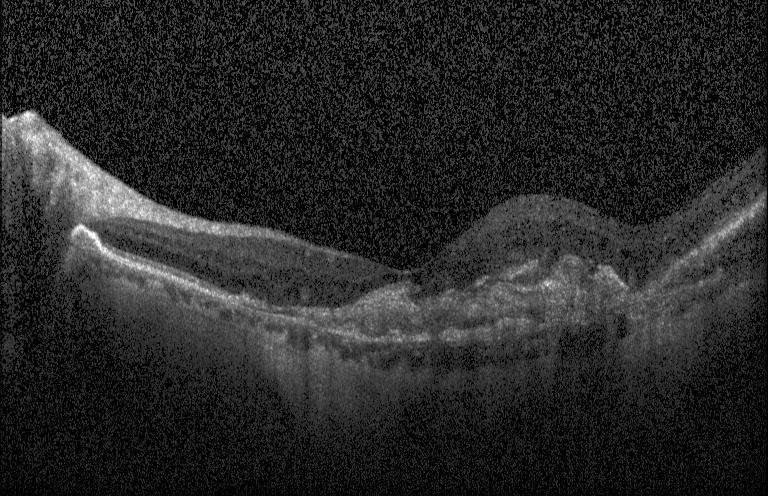

Spectral-domain OCT B-scan: a choroidal neovascular membrane.